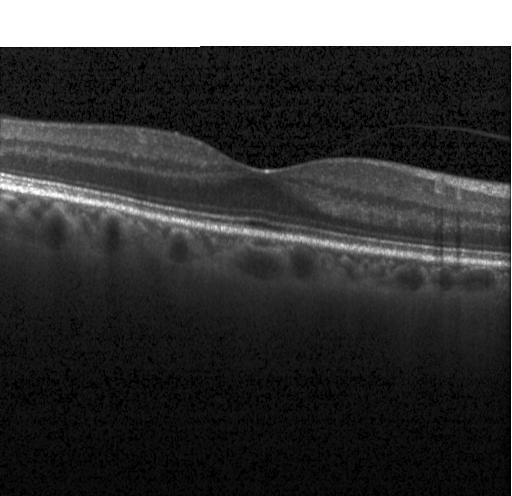 Spectral-domain optical coherence tomography; optical coherence tomography scan; macular scan; instrument: Heidelberg Spectralis
Assessment: neither choroidal neovascularization, diabetic macular edema, nor drusen.